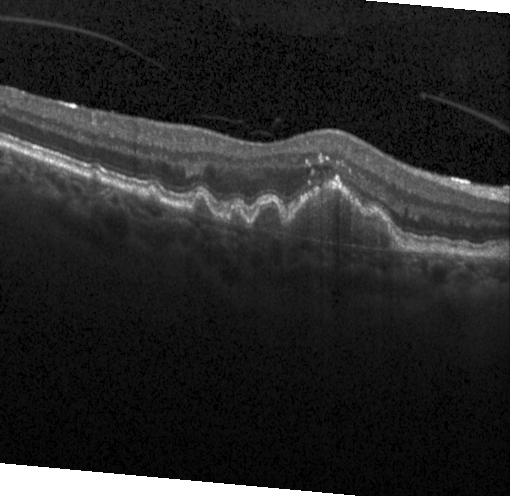 Diagnosis: a choroidal neovascular membrane.